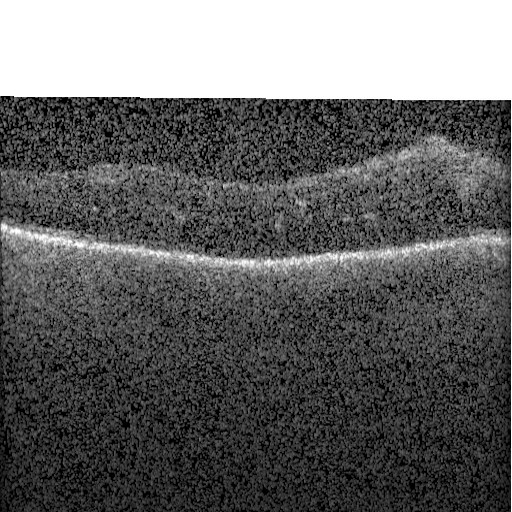 Assessment: diabetic macular edema.